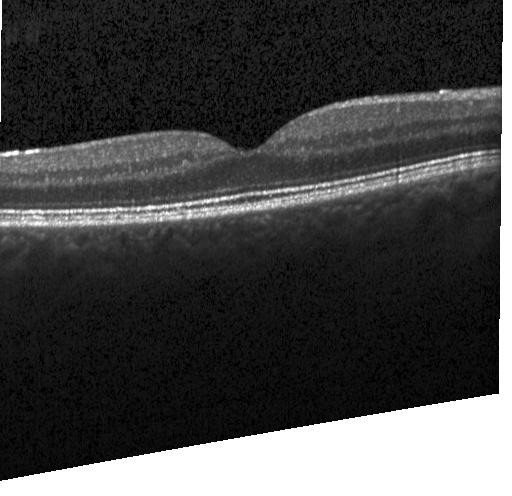 Finding: no CNV, DME, or drusen.